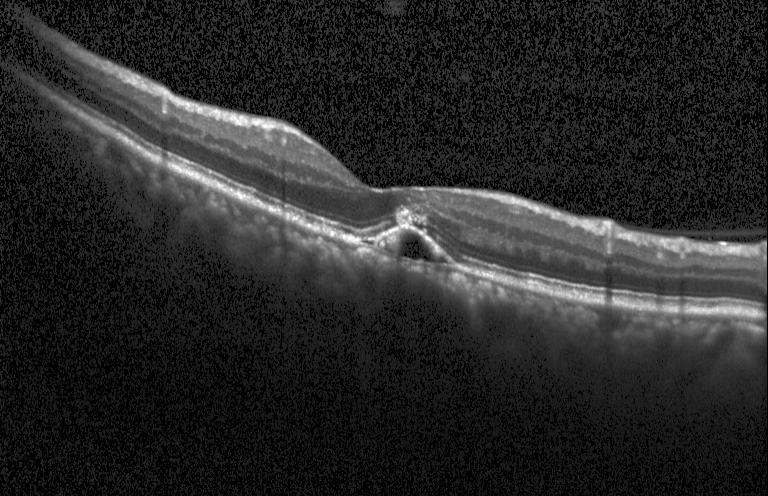

Heidelberg Spectralis; spectral-domain OCT; centered on the fovea; OCT B-scan. A choroidal neovascular membrane.